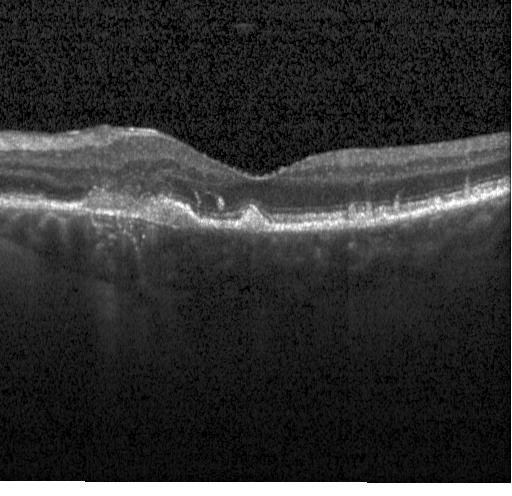
Optical coherence tomography B-scan. Impression: a choroidal neovascular membrane.